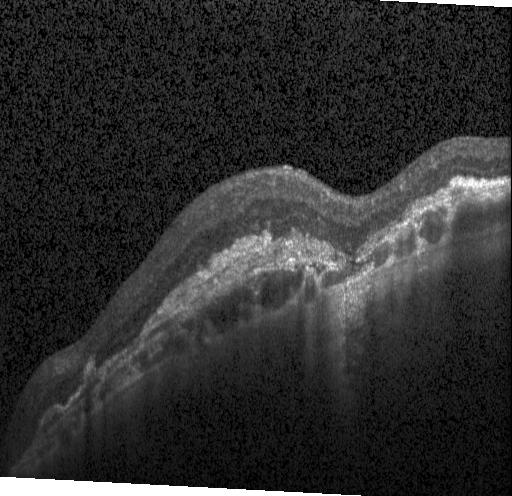 Through the macula · spectral-domain optical coherence tomography · OCT line scan — OCT finding: a choroidal neovascular membrane.